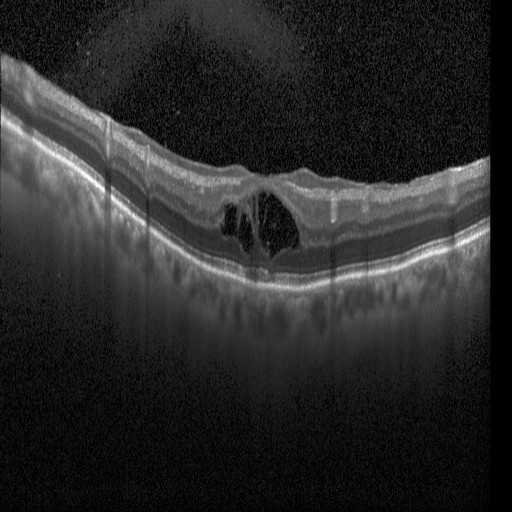

Retinal OCT cross-section; through the macula. Diabetic macular edema (DME).